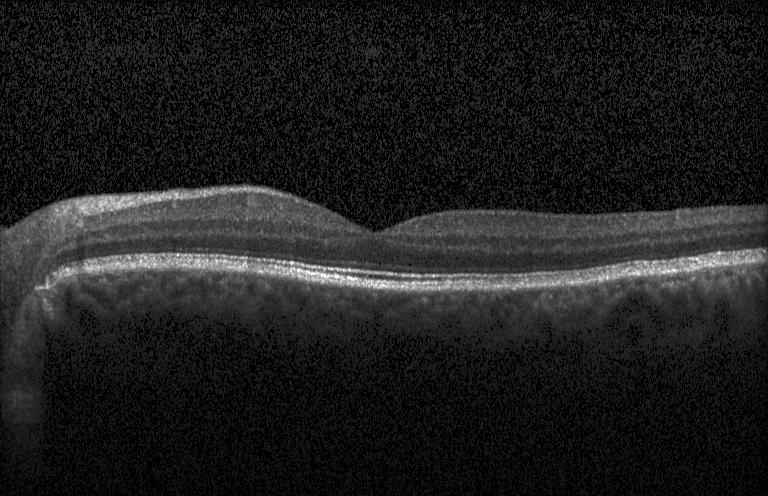 This B-scan demonstrates no choroidal neovascularization, diabetic macular edema, or drusen.